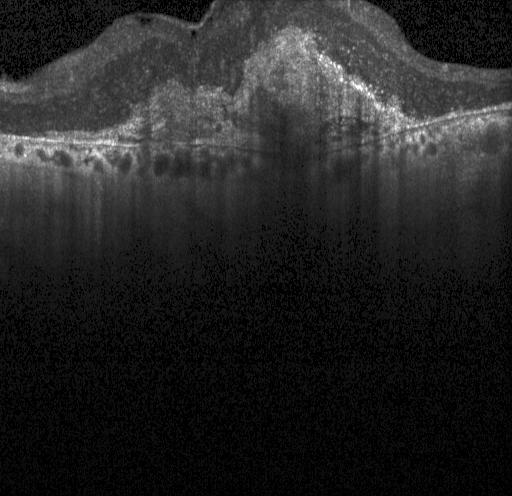 Optical coherence tomography scan.
Diagnosis: a choroidal neovascular membrane.